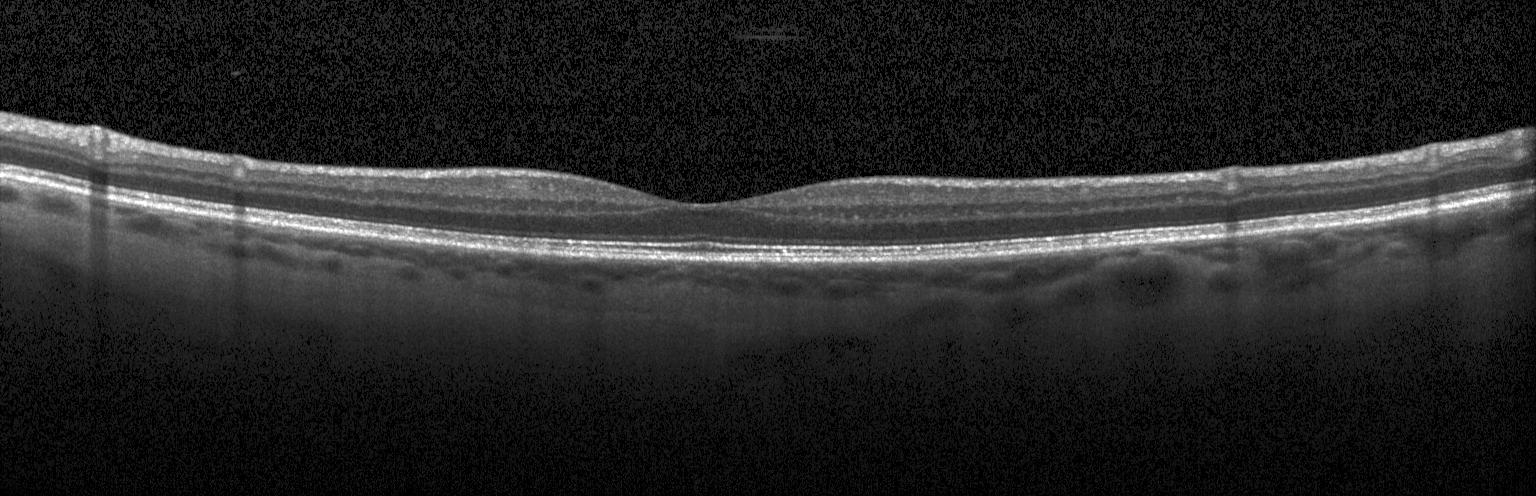

Assessment: no evidence of choroidal neovascularization, diabetic macular edema, or drusen.